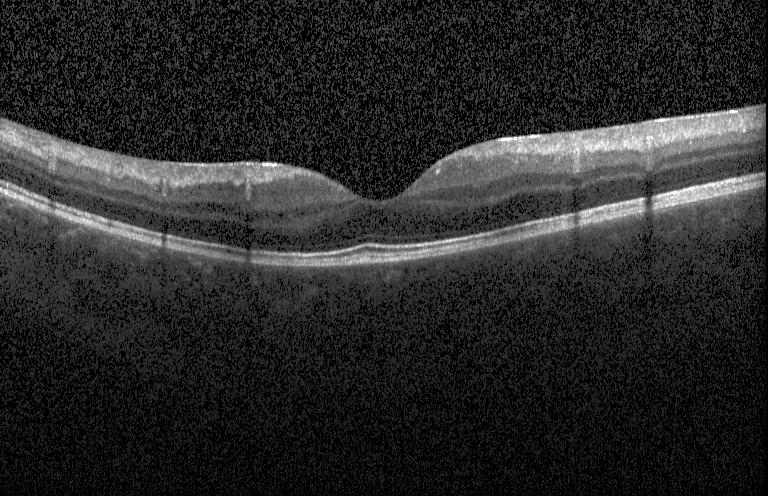

OCT scan showing no evidence of CNV, DME, or drusen.